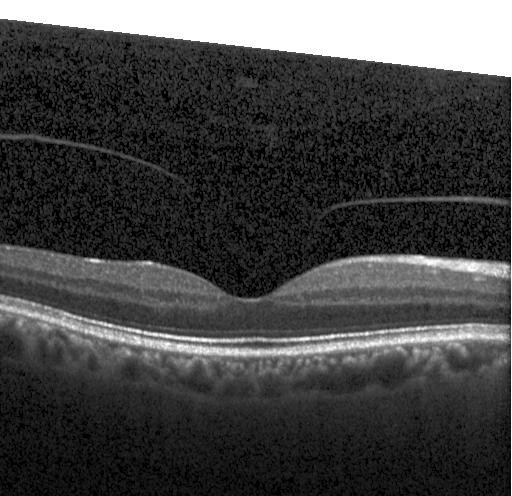

Centered on the fovea. Optical coherence tomography scan. Heidelberg Spectralis OCT system. Spectral-domain optical coherence tomography.
Assessment: neither choroidal neovascularization, diabetic macular edema, nor drusen.